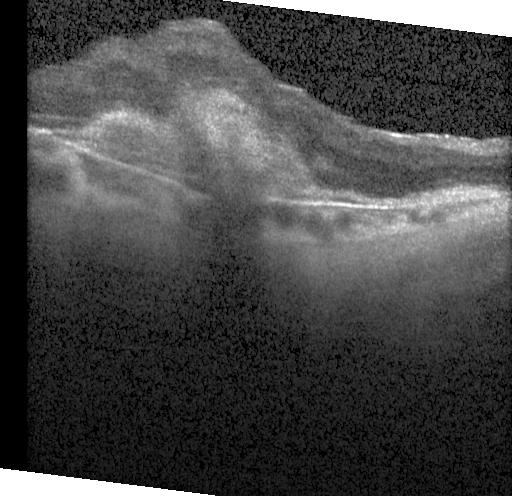

Spectral-domain optical coherence tomography. Retinal OCT cross-section.
The scan shows CNV.